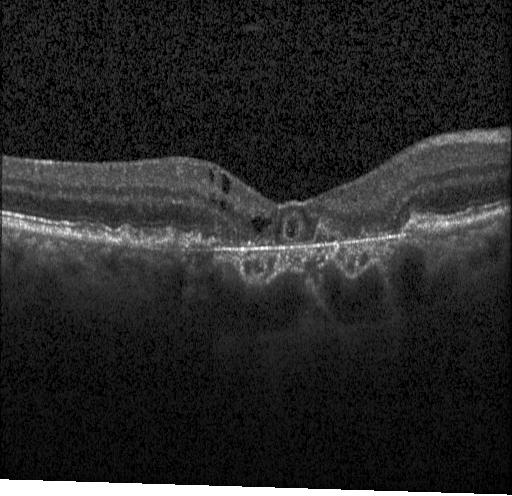
Diagnosis: CNV.